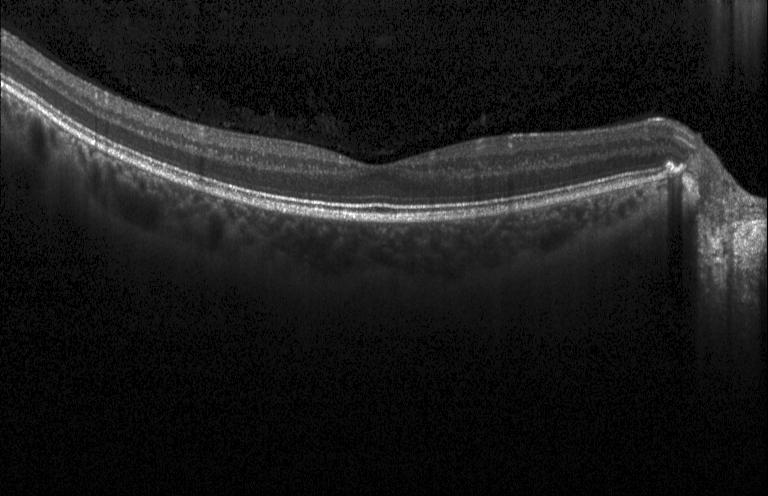 Retinal OCT B-scan
Assessment: no choroidal neovascularization, no diabetic macular edema, and no drusen.